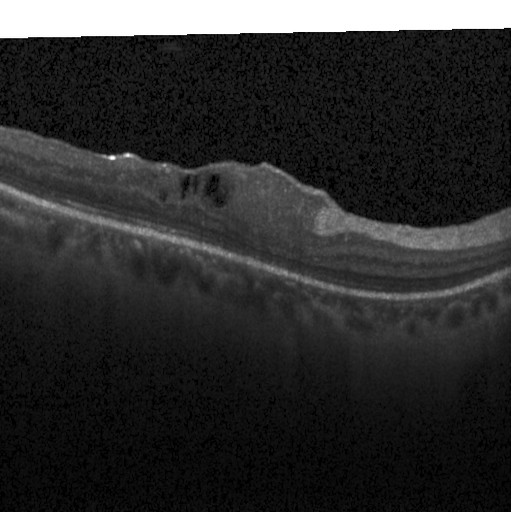 Optical coherence tomography B-scan — OCT finding: diabetic macular edema (DME).